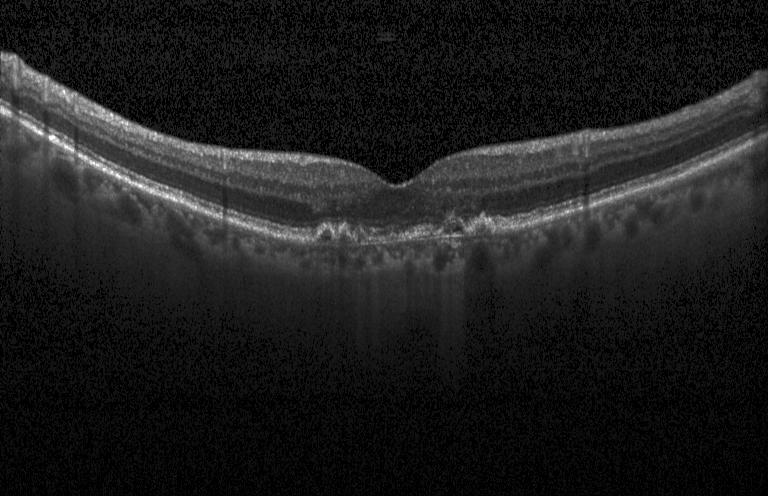 Diagnosis: drusen.